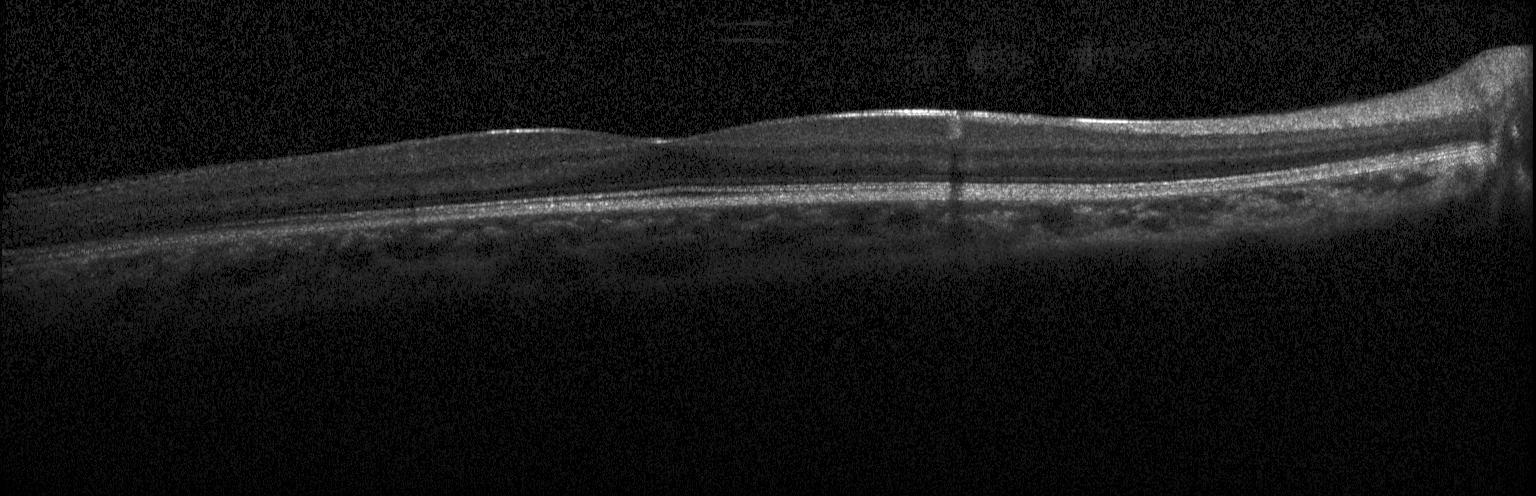 Spectral-domain optical coherence tomography, optical coherence tomography B-scan, fovea-centered. Impression: neither choroidal neovascularization, diabetic macular edema, nor drusen.